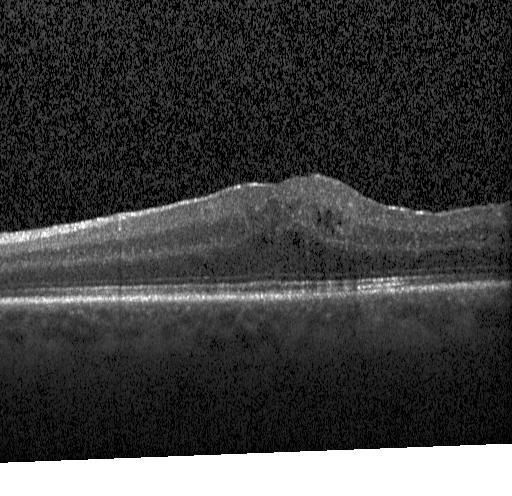 Dx: diabetic macular edema.